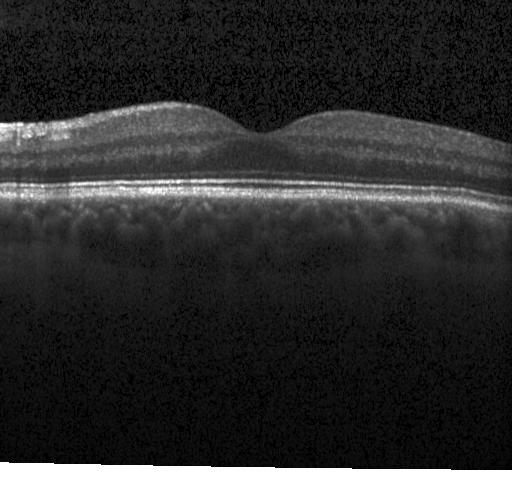
Spectral-domain OCT · macular scan · retinal OCT cross-section · acquired on a Heidelberg Spectralis.
Impression: no evidence of choroidal neovascularization, diabetic macular edema, or drusen.